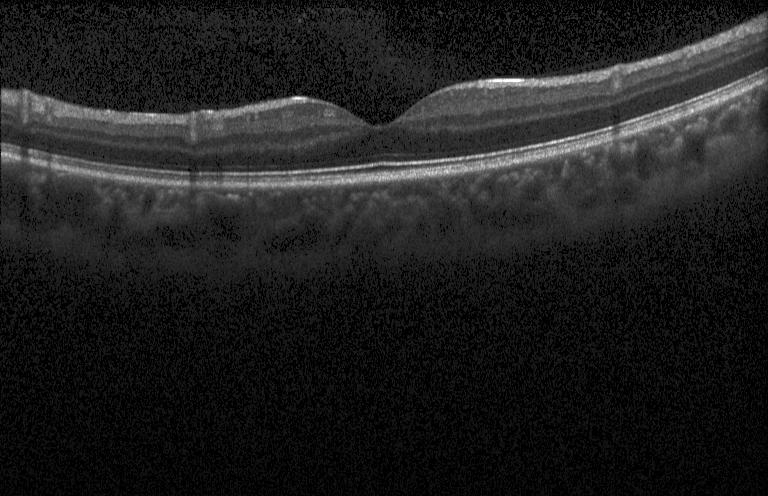 Assessment: no choroidal neovascularization, no diabetic macular edema, and no drusen.